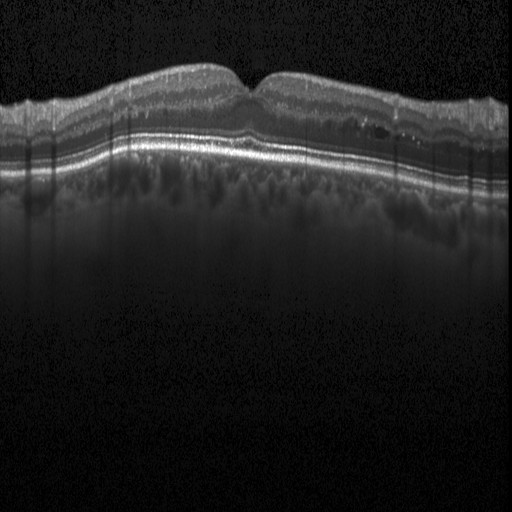

DME.